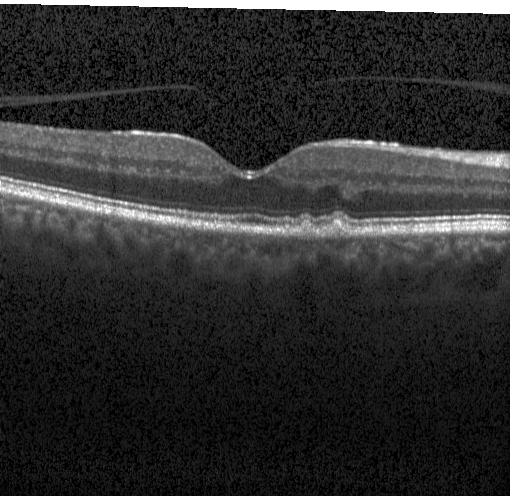
OCT line scan
Diagnosis: drusen.